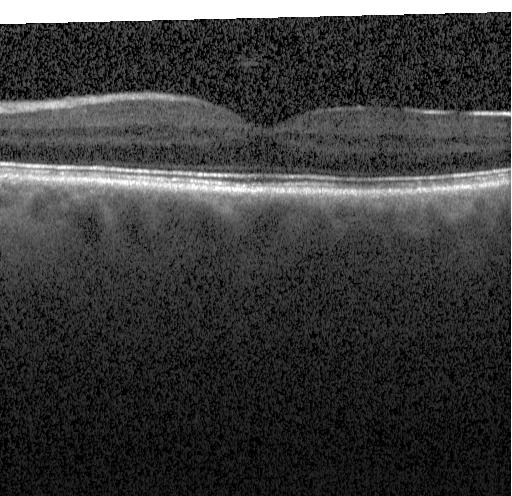
Finding: no choroidal neovascularization, no diabetic macular edema, and no drusen.